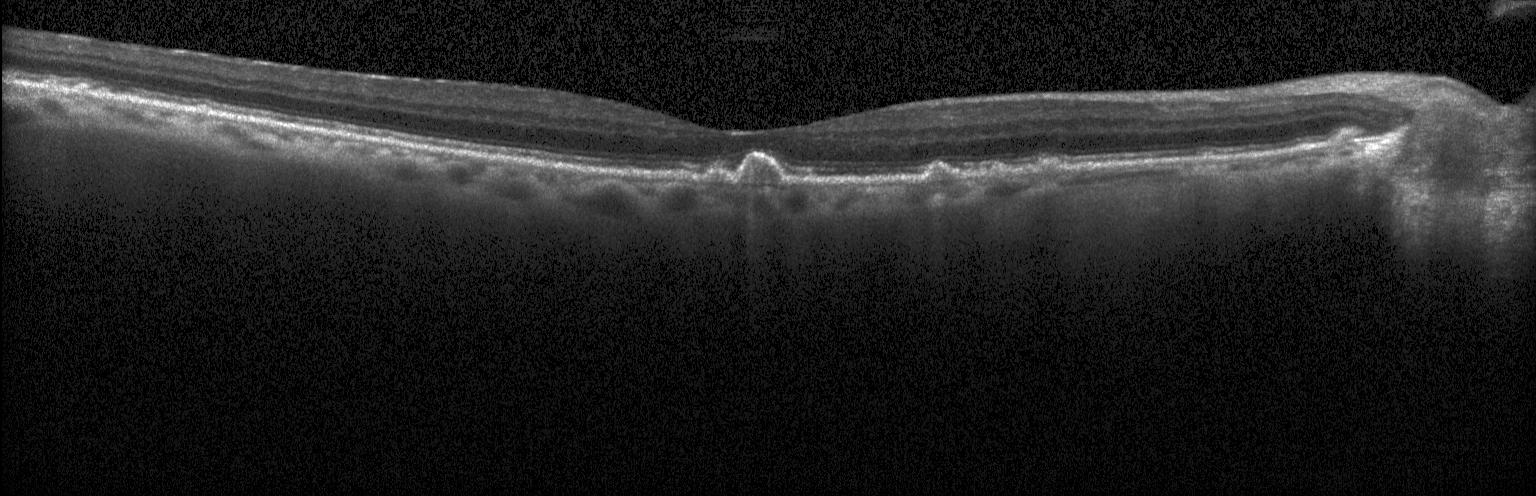

Impression: drusen.